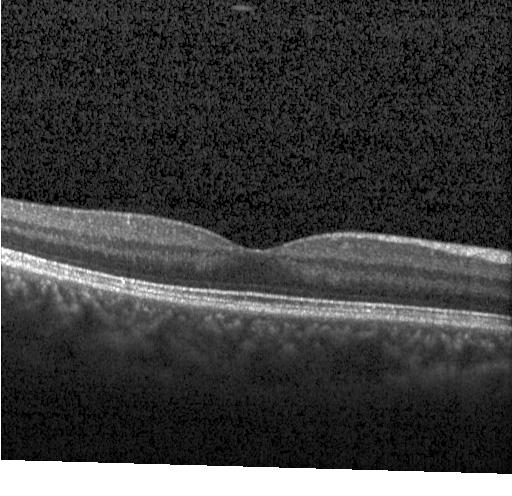 OCT scan showing neither choroidal neovascularization, diabetic macular edema, nor drusen.